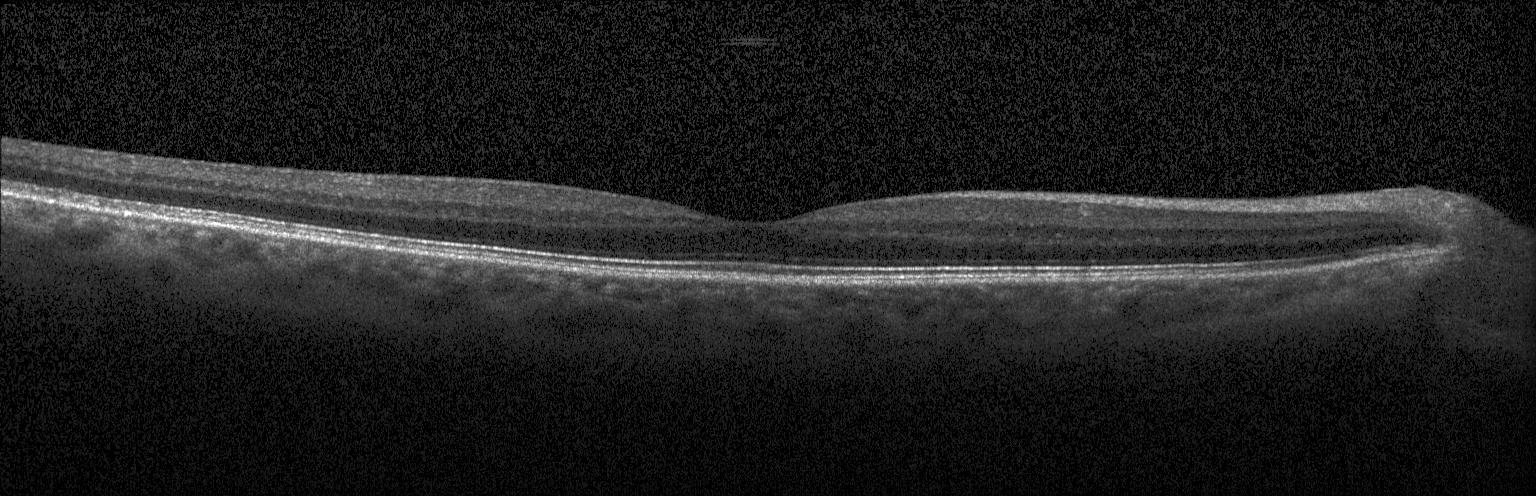

OCT line scan. This B-scan demonstrates no choroidal neovascularization, no diabetic macular edema, and no drusen.